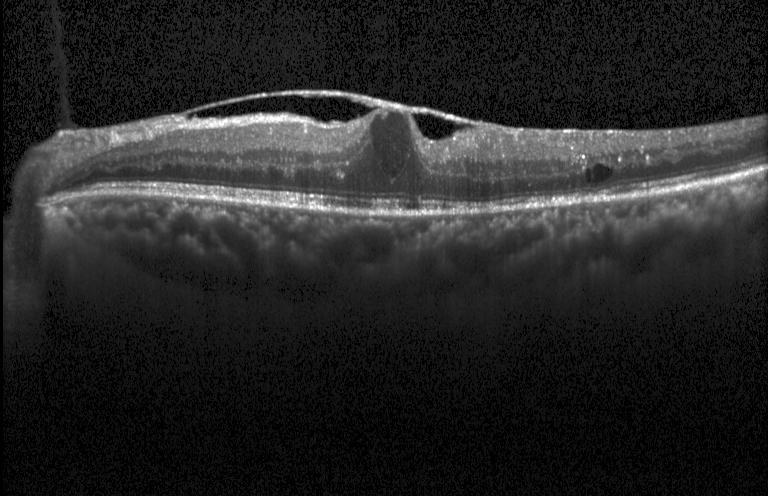

Optical coherence tomography scan. Impression: diabetic macular edema.